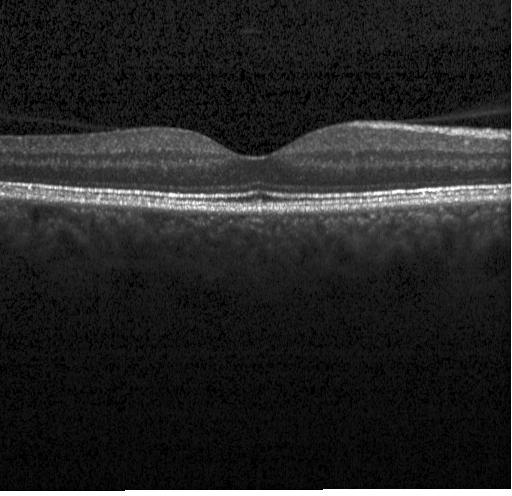 Retinal OCT cross-section — Impression: no choroidal neovascularization, diabetic macular edema, or drusen.